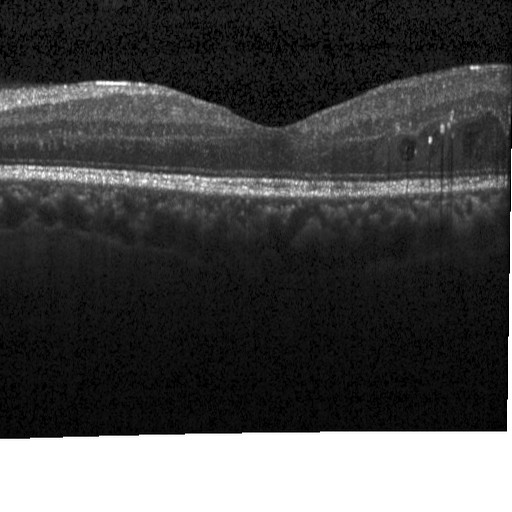 SD-OCT, Heidelberg Spectralis OCT system, optical coherence tomography B-scan.
Impression: diabetic macular edema (DME).